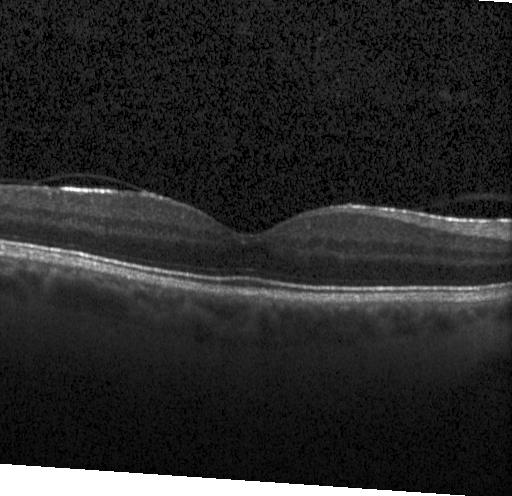 OCT line scan. OCT finding: neither choroidal neovascularization, diabetic macular edema, nor drusen.